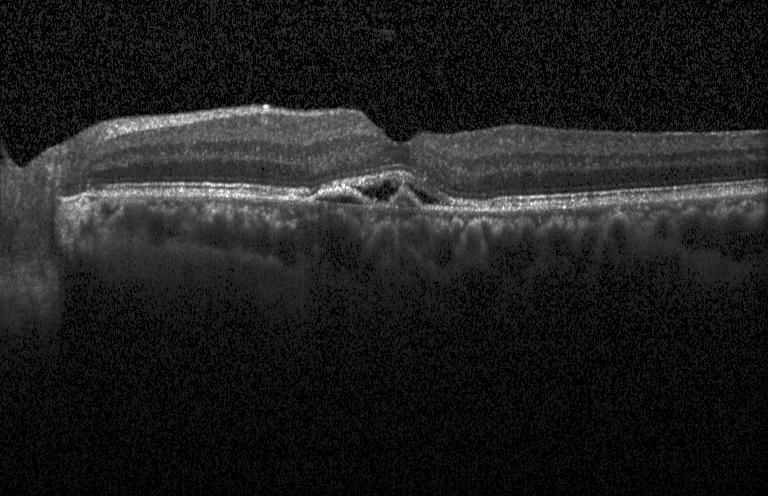 This B-scan demonstrates a choroidal neovascular membrane.